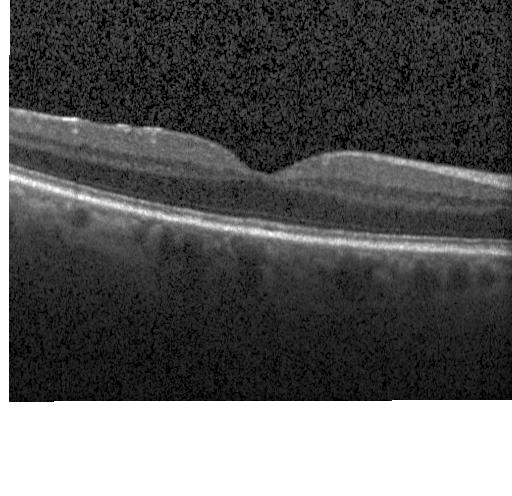
Macular scan; OCT line scan; Heidelberg Spectralis. This B-scan demonstrates neither choroidal neovascularization, diabetic macular edema, nor drusen.